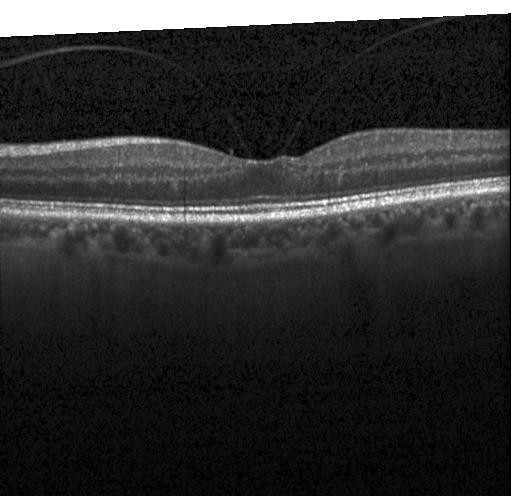

Heidelberg Spectralis OCT system · optical coherence tomography B-scan · SD-OCT · horizontal scan through the fovea — Impression: neither choroidal neovascularization, diabetic macular edema, nor drusen.